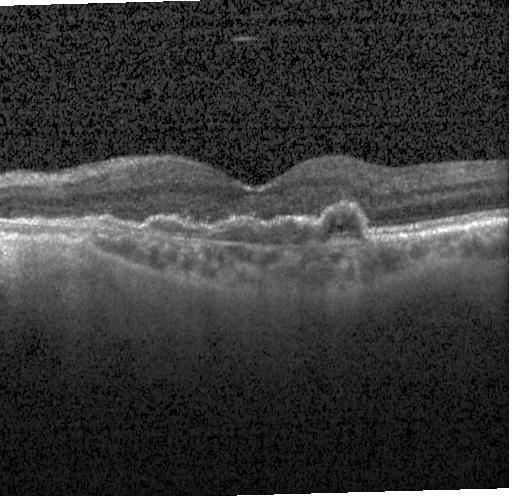 Optical coherence tomography B-scan.
This B-scan demonstrates a choroidal neovascular membrane.